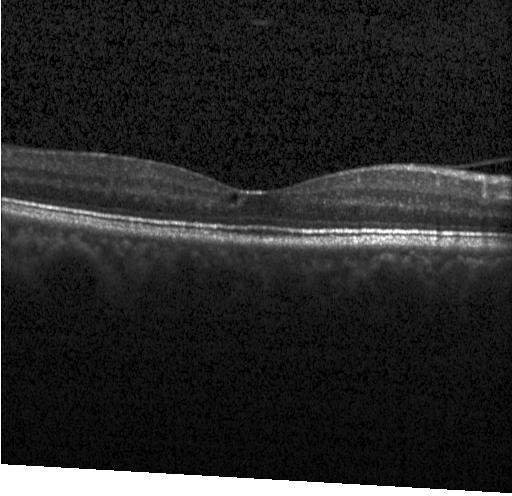 Diagnosis: diabetic macular edema.